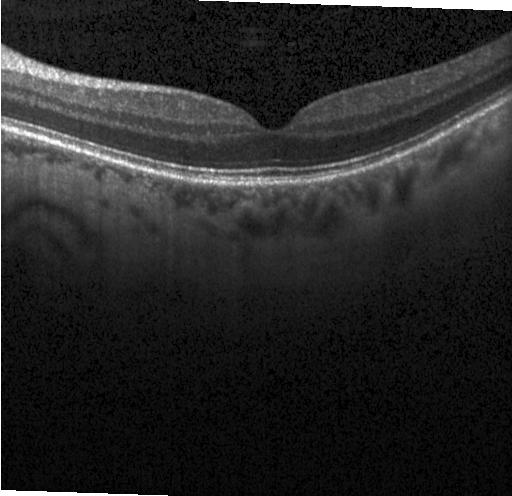 No CNV, no DME, and no drusen.